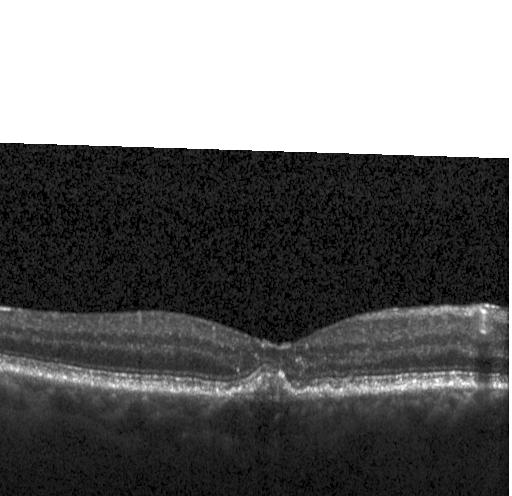

Macular scan, spectral-domain optical coherence tomography, optical coherence tomography B-scan, Heidelberg Spectralis
Assessment: sub-RPE drusenoid deposits.